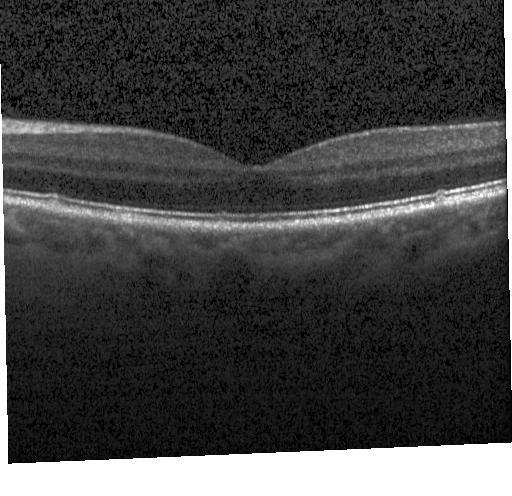

OCT B-scan; fovea-centered; Heidelberg Spectralis OCT system; spectral-domain OCT.
Dx: sub-RPE drusenoid deposits.